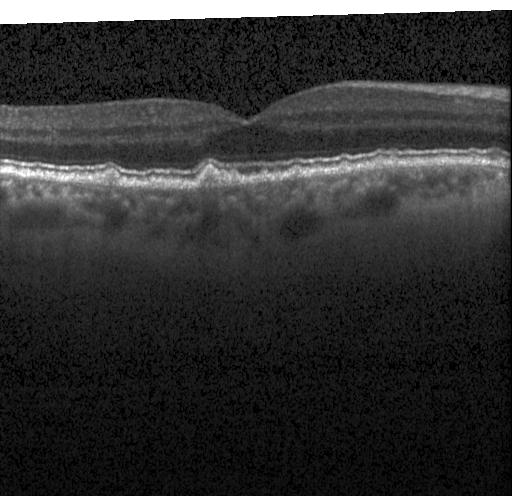

Drusen.